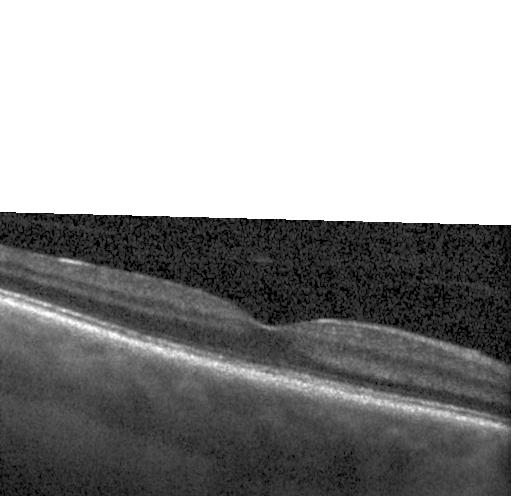
Spectral-domain OCT. Heidelberg Spectralis OCT system. Fovea-centered. Retinal OCT B-scan
Macular OCT: no choroidal neovascularization, diabetic macular edema, or drusen.